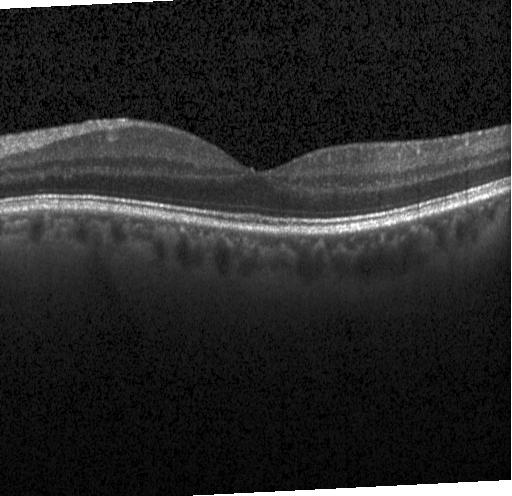

Diagnosis: no choroidal neovascularization, diabetic macular edema, or drusen.